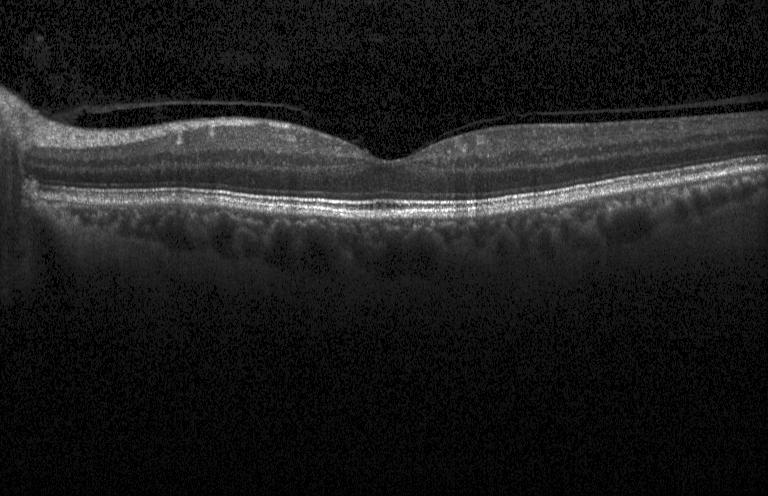
Retinal OCT cross-section.
Macular OCT: no evidence of CNV, DME, or drusen.